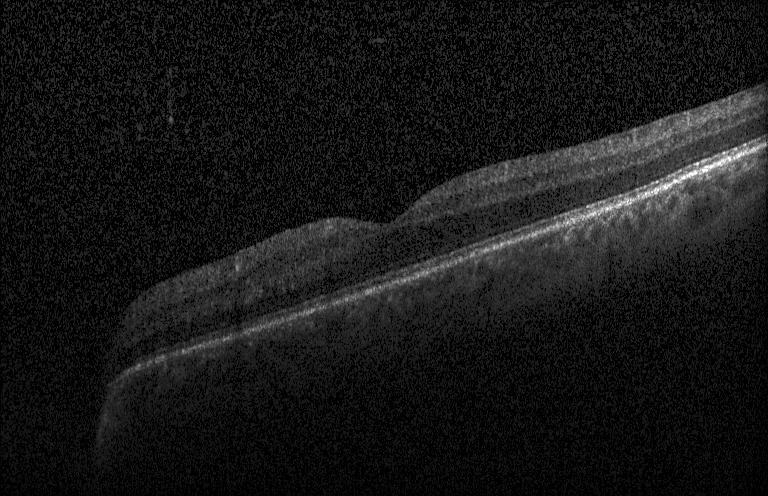
OCT B-scan; Heidelberg Spectralis — No CNV, no DME, and no drusen.